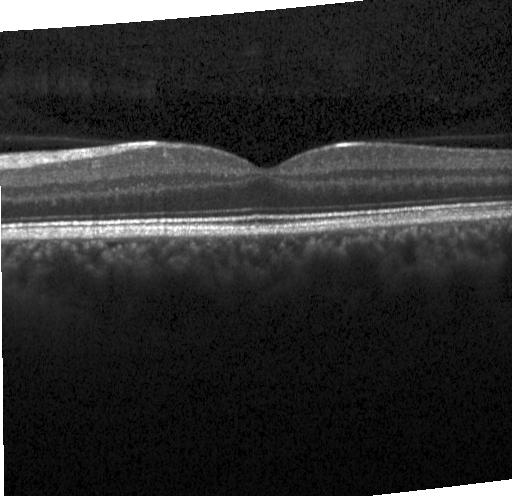 Retinal OCT B-scan
Diagnosis: no CNV, no DME, and no drusen.